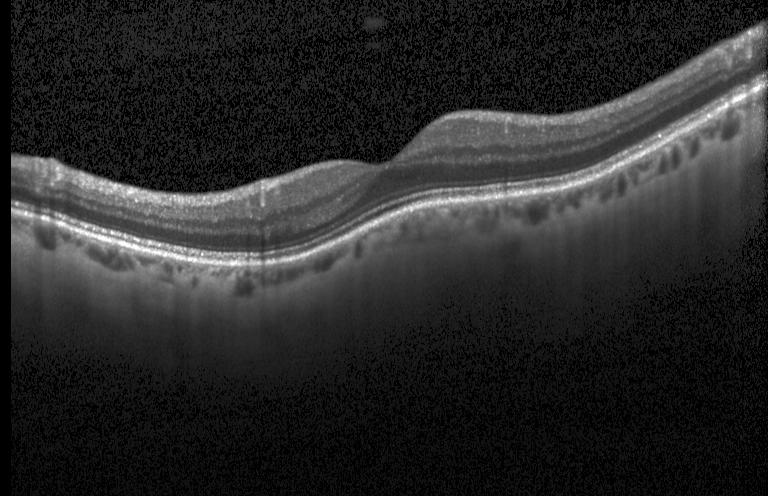
OCT scan showing no choroidal neovascularization, diabetic macular edema, or drusen.